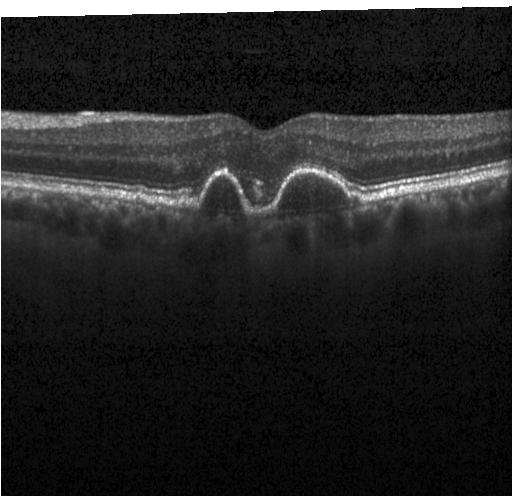
OCT line scan. Spectral-domain optical coherence tomography. Fovea-centered. Instrument: Heidelberg Spectralis.
Assessment: a choroidal neovascular membrane.